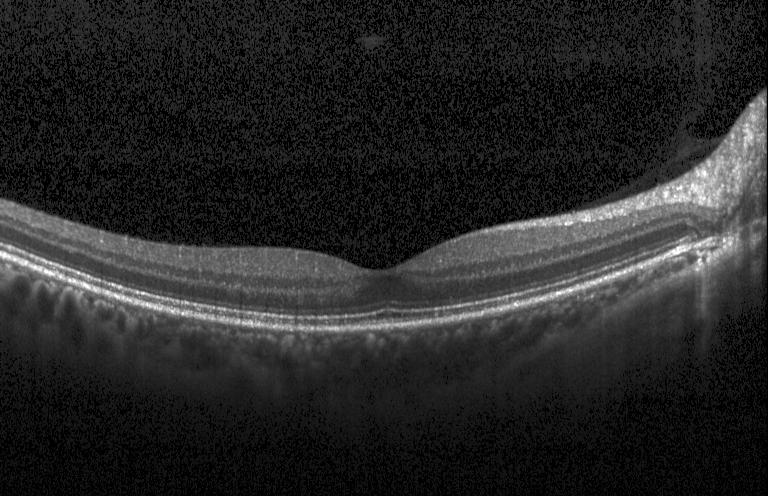
Instrument: Heidelberg Spectralis · optical coherence tomography scan. Impression: no evidence of choroidal neovascularization, diabetic macular edema, or drusen.